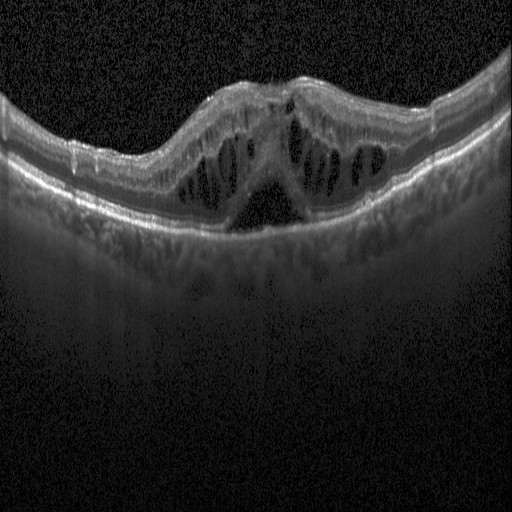

Macular scan · OCT line scan · instrument: Heidelberg Spectralis · spectral-domain optical coherence tomography
Macular OCT: DME.